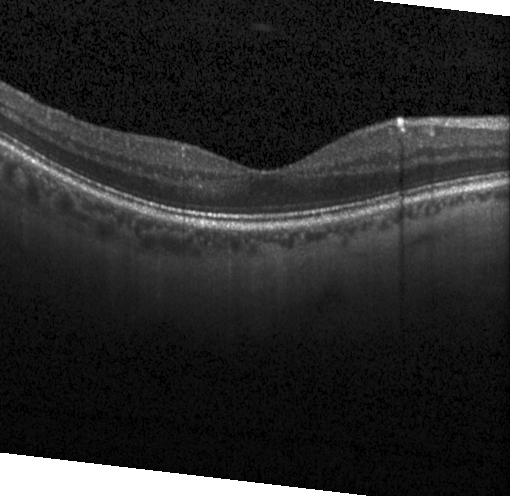
Macular OCT demonstrating no choroidal neovascularization, diabetic macular edema, or drusen.